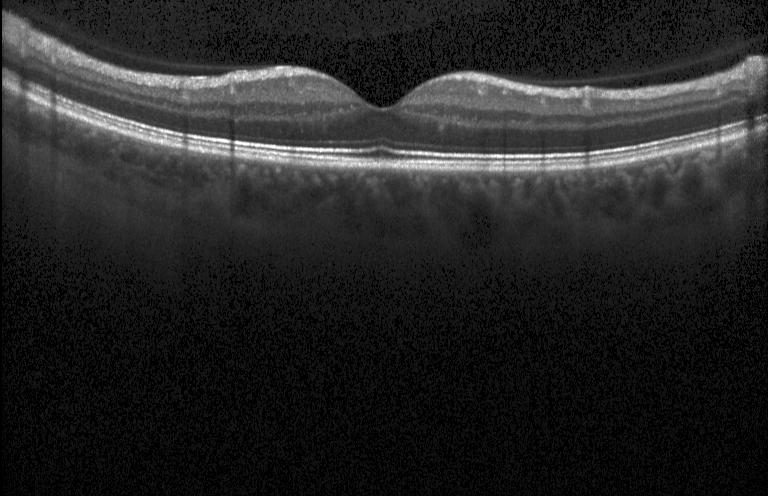 Dx: no evidence of choroidal neovascularization, diabetic macular edema, or drusen.